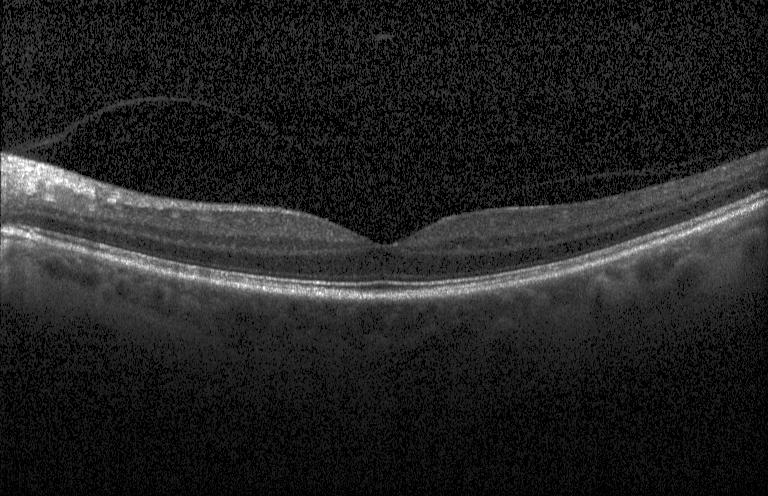
Heidelberg Spectralis OCT system · retinal OCT B-scan
Impression: neither CNV, DME, nor drusen.